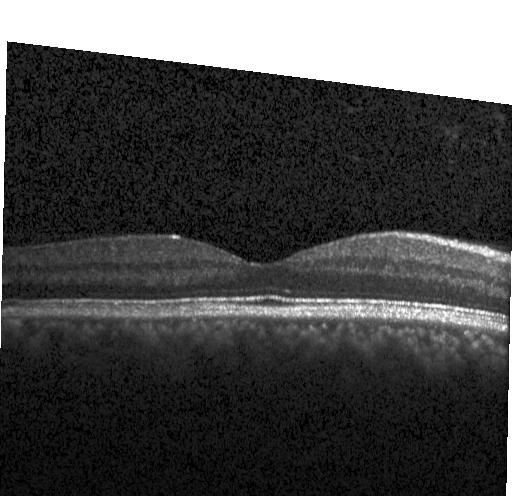

Assessment: neither choroidal neovascularization, diabetic macular edema, nor drusen.